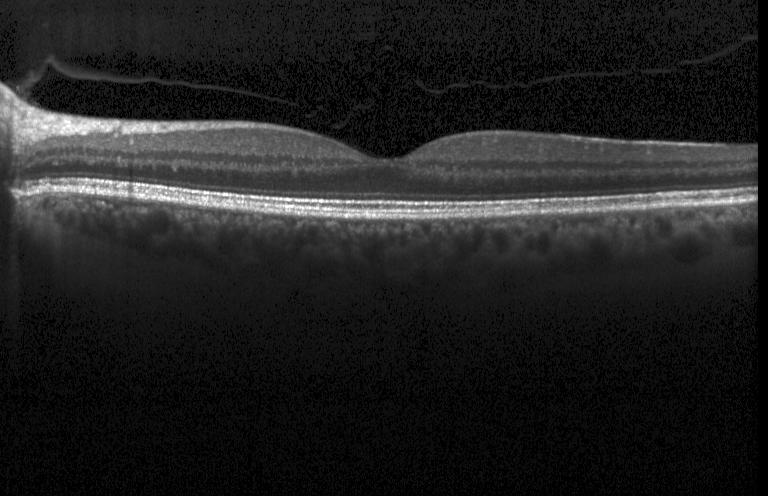 Retinal OCT B-scan. Finding: no CNV, DME, or drusen.